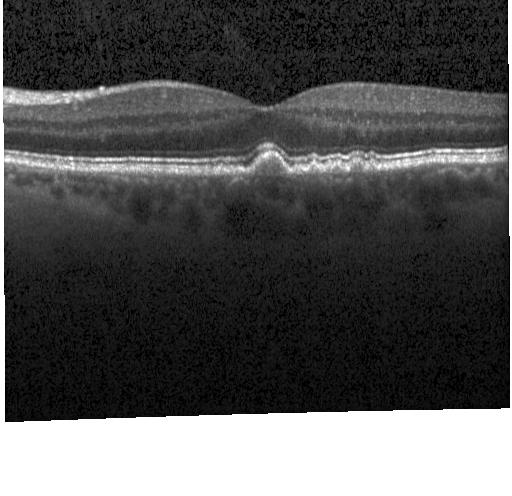

Optical coherence tomography B-scan, Heidelberg Spectralis, SD-OCT — Impression: multiple drusen.